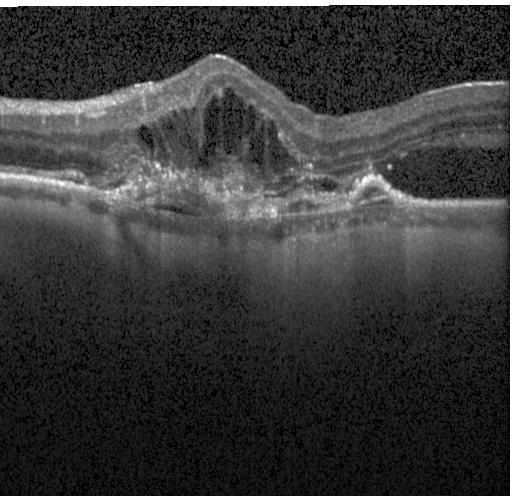
Spectral-domain OCT. Retinal OCT B-scan. Through the macula. Diagnosis: a choroidal neovascular membrane.